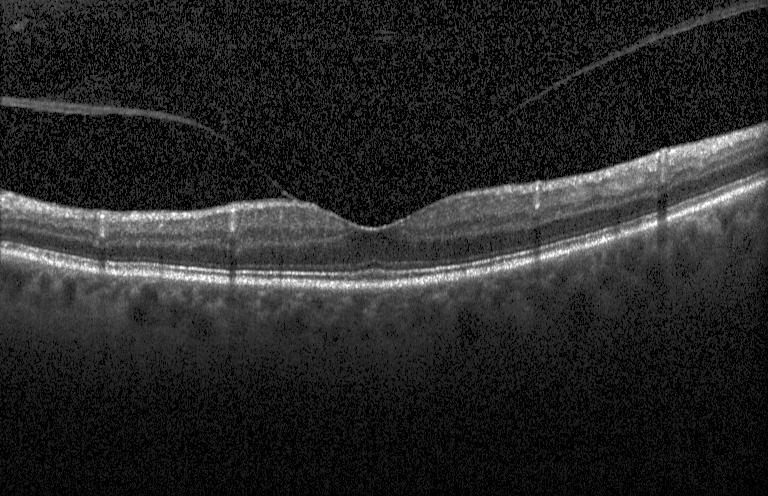
Optical coherence tomography B-scan.
OCT finding: no choroidal neovascularization, diabetic macular edema, or drusen.